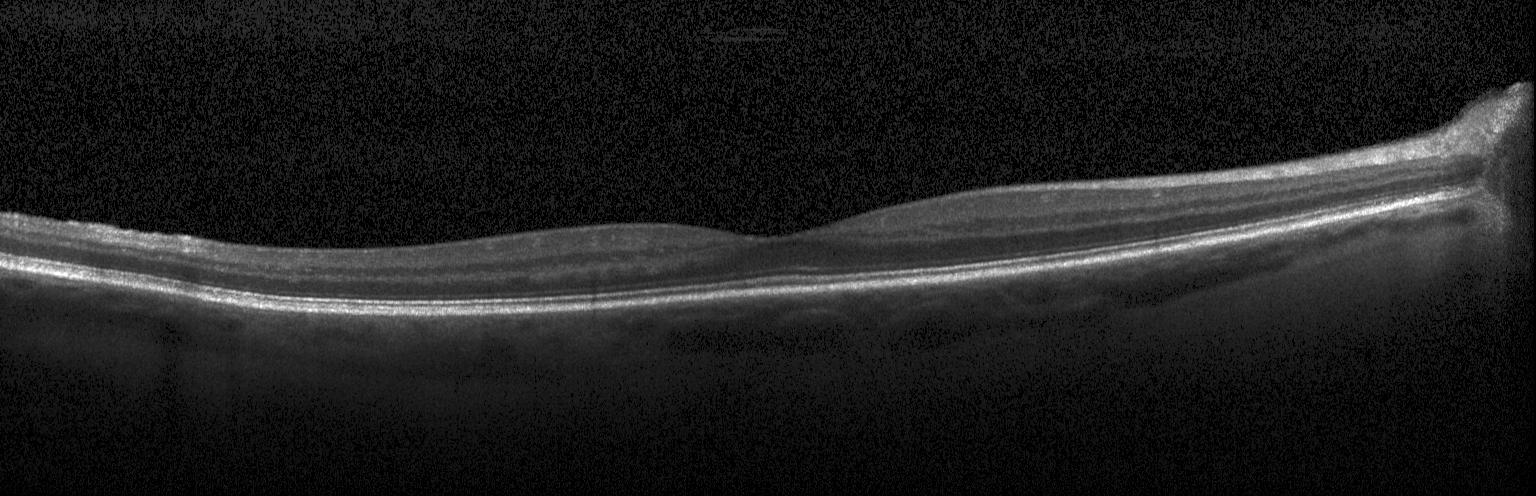

This B-scan demonstrates no choroidal neovascularization, diabetic macular edema, or drusen.